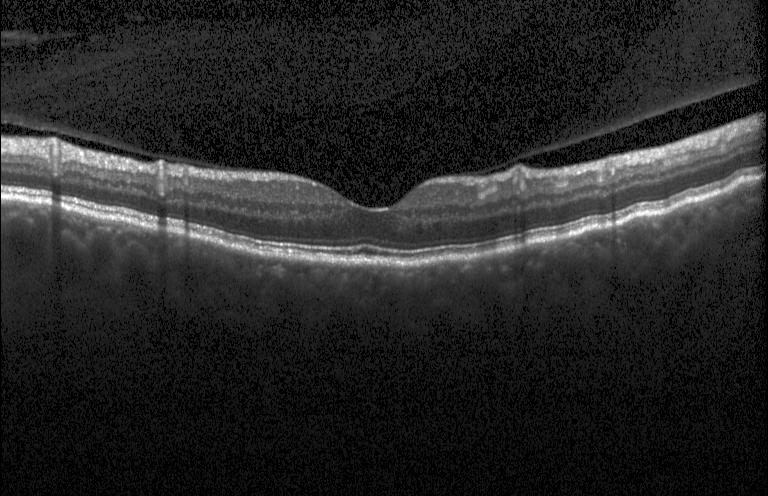

Impression: neither choroidal neovascularization, diabetic macular edema, nor drusen.